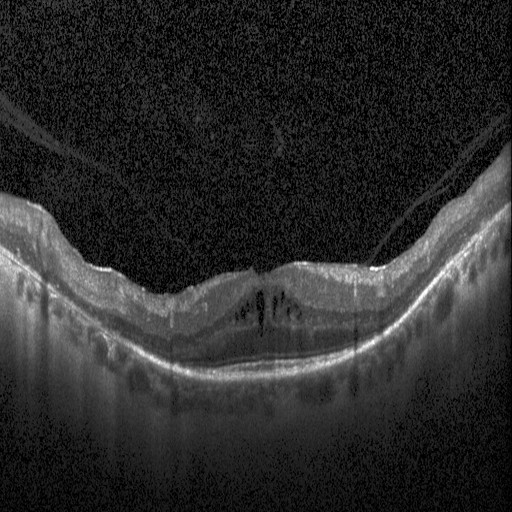 Spectral-domain optical coherence tomography, macular scan, OCT line scan, instrument: Heidelberg Spectralis.
DME.